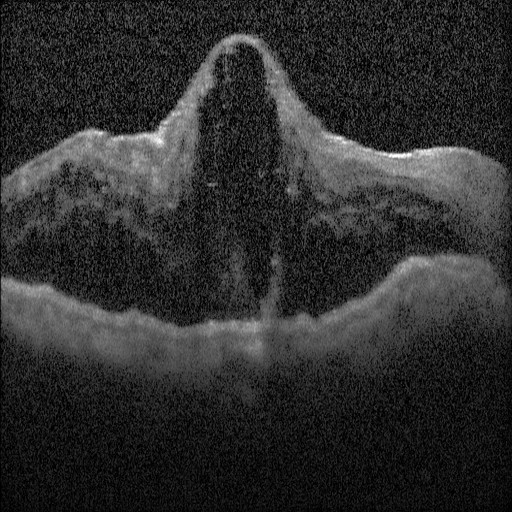
Horizontal scan through the fovea, instrument: Heidelberg Spectralis, OCT line scan — Dx: diabetic macular edema.